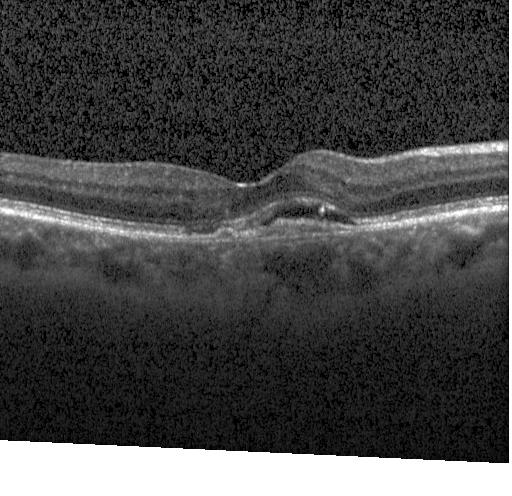

SD-OCT · OCT line scan. Dx: choroidal neovascularization (CNV).